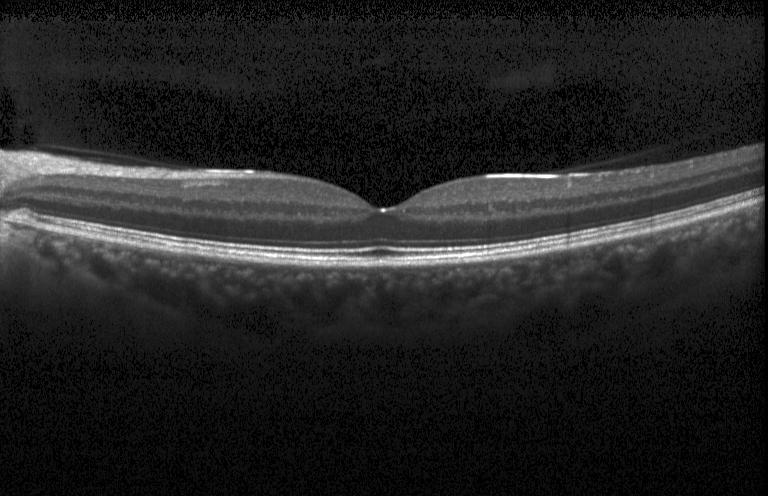
Dx: no evidence of choroidal neovascularization, diabetic macular edema, or drusen.